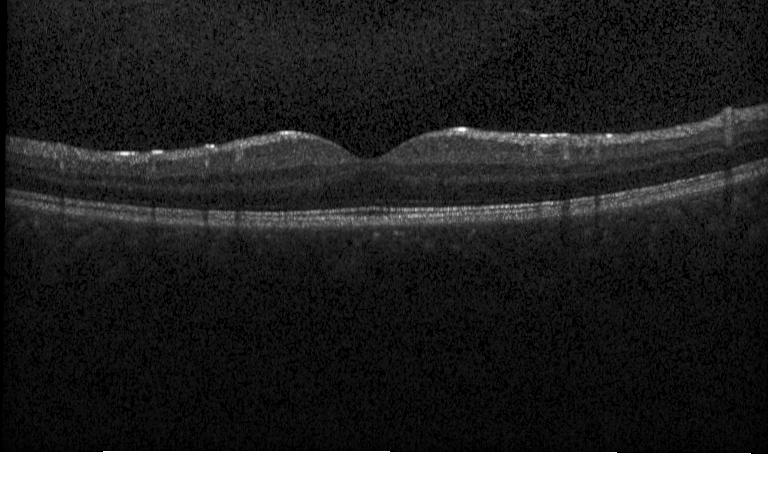

Optical coherence tomography scan · spectral-domain OCT
Macular OCT: no choroidal neovascularization, diabetic macular edema, or drusen.